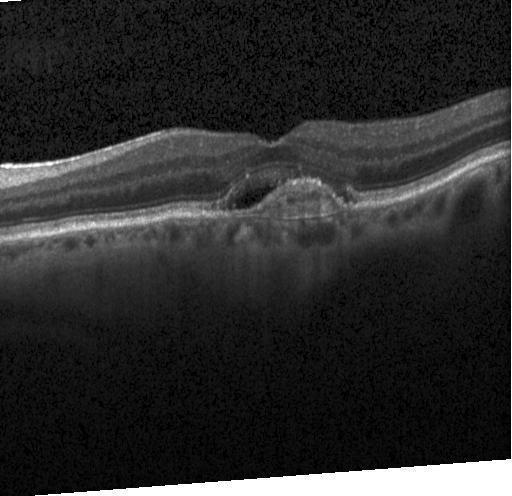 Spectral-domain optical coherence tomography; macular scan; optical coherence tomography B-scan
Finding: a choroidal neovascular membrane.